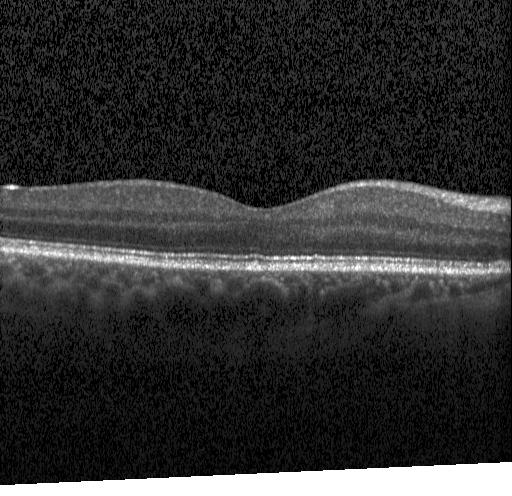
Horizontal scan through the fovea; optical coherence tomography B-scan; instrument: Heidelberg Spectralis — No choroidal neovascularization, diabetic macular edema, or drusen.